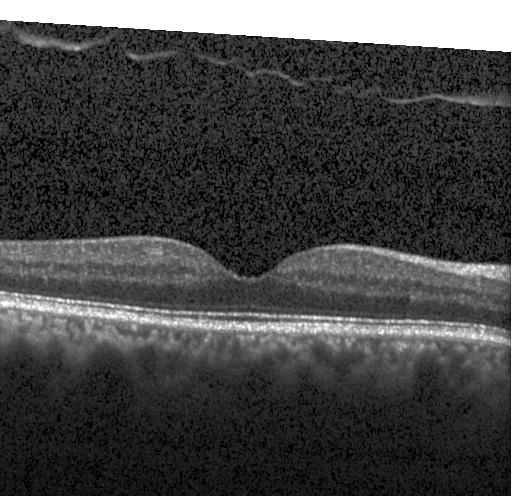 Macular scan · Heidelberg Spectralis OCT system · optical coherence tomography B-scan.
Assessment: no choroidal neovascularization, diabetic macular edema, or drusen.